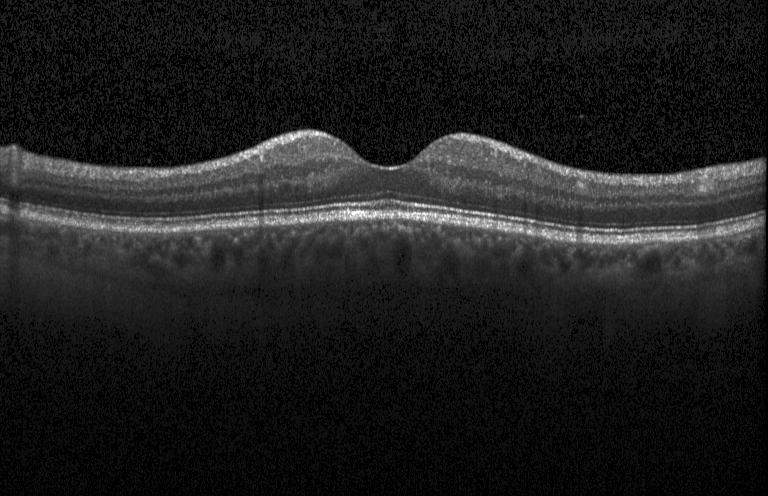
Instrument: Heidelberg Spectralis. Fovea-centered. OCT line scan. The scan shows neither CNV, DME, nor drusen.